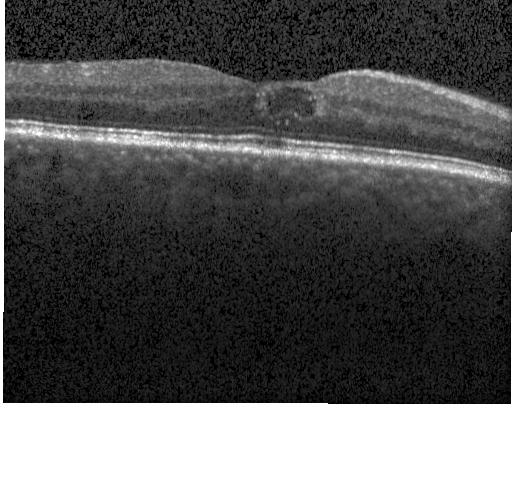

OCT B-scan; Heidelberg Spectralis OCT system. Finding: diabetic macular edema.